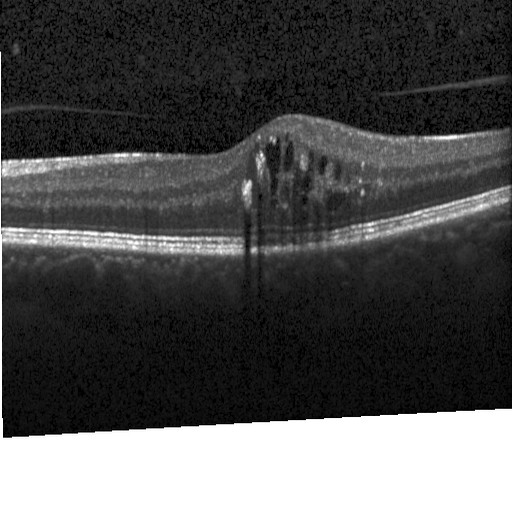

Retinal OCT B-scan; horizontal scan through the fovea; Heidelberg Spectralis; spectral-domain optical coherence tomography.
Impression: DME.